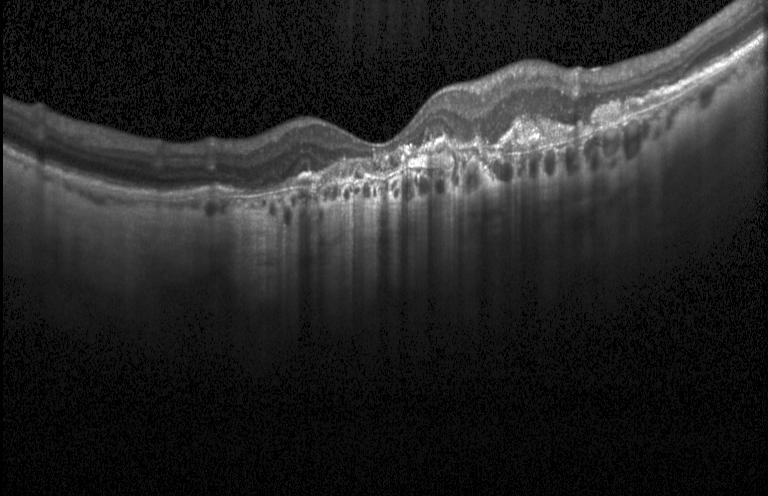 Spectral-domain OCT; optical coherence tomography B-scan
This B-scan demonstrates CNV.